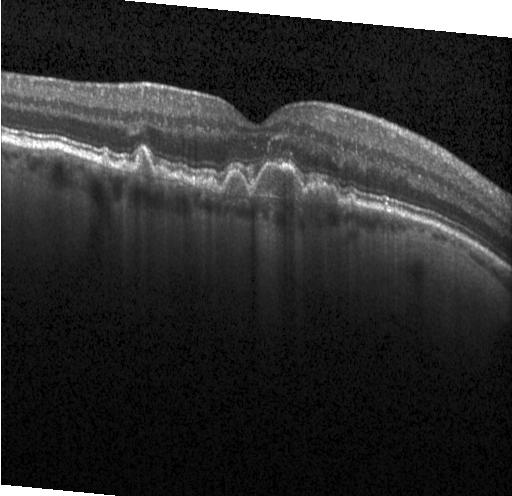 Macular OCT: multiple drusen.